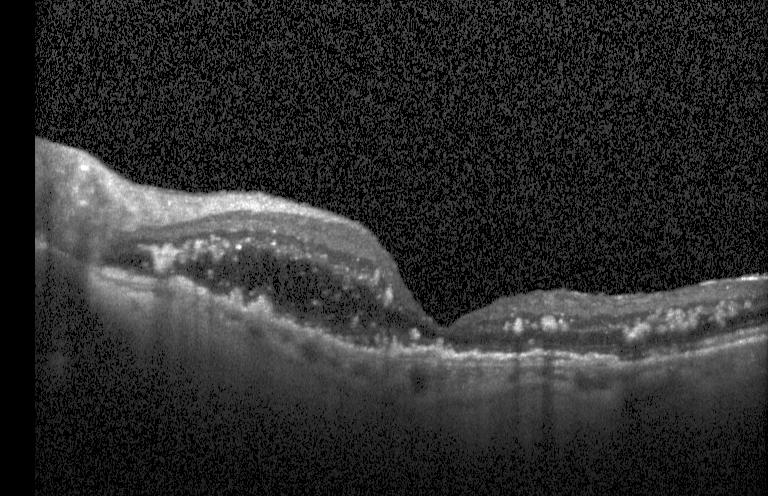
Heidelberg Spectralis, spectral-domain optical coherence tomography, horizontal scan through the fovea, retinal OCT B-scan.
Finding: choroidal neovascularization (CNV).